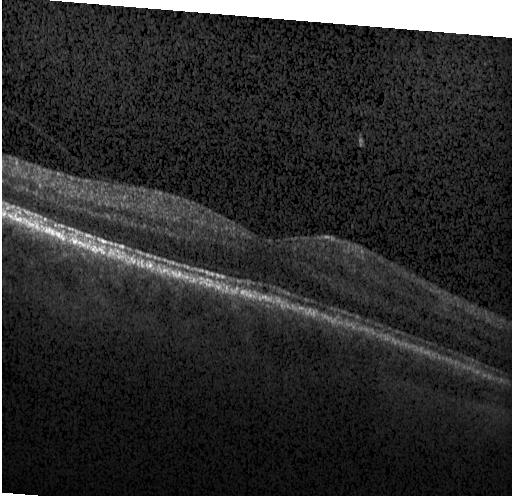 Heidelberg Spectralis OCT system. Spectral-domain OCT. Retinal OCT B-scan — Dx: neither CNV, DME, nor drusen.